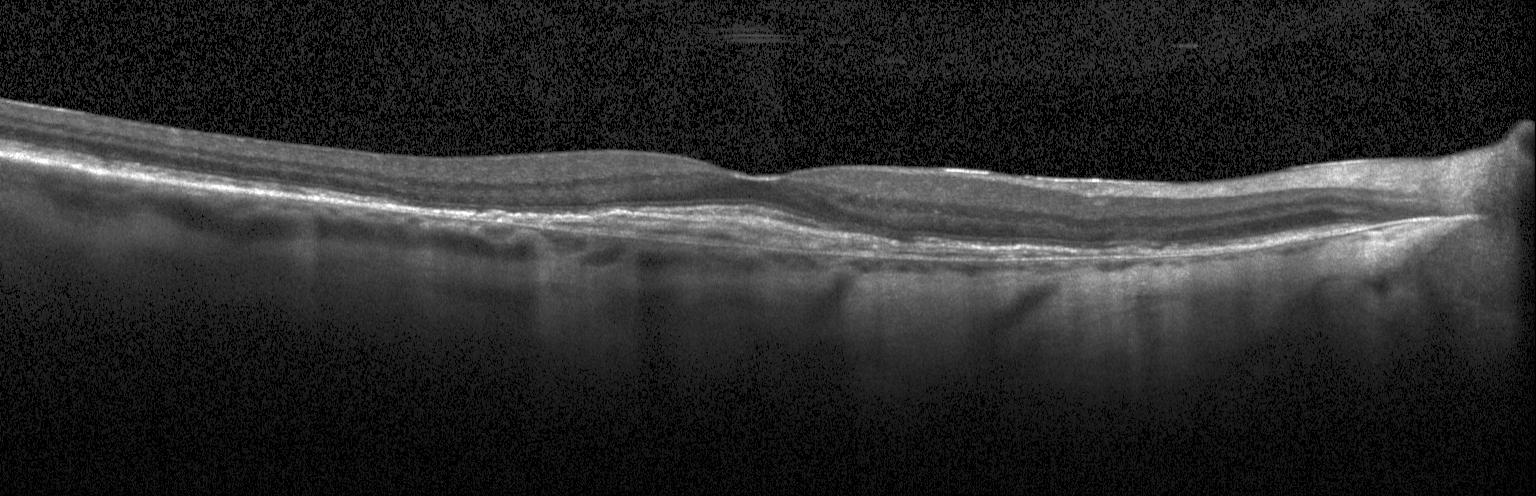

Optical coherence tomography B-scan.
This B-scan demonstrates choroidal neovascularization.